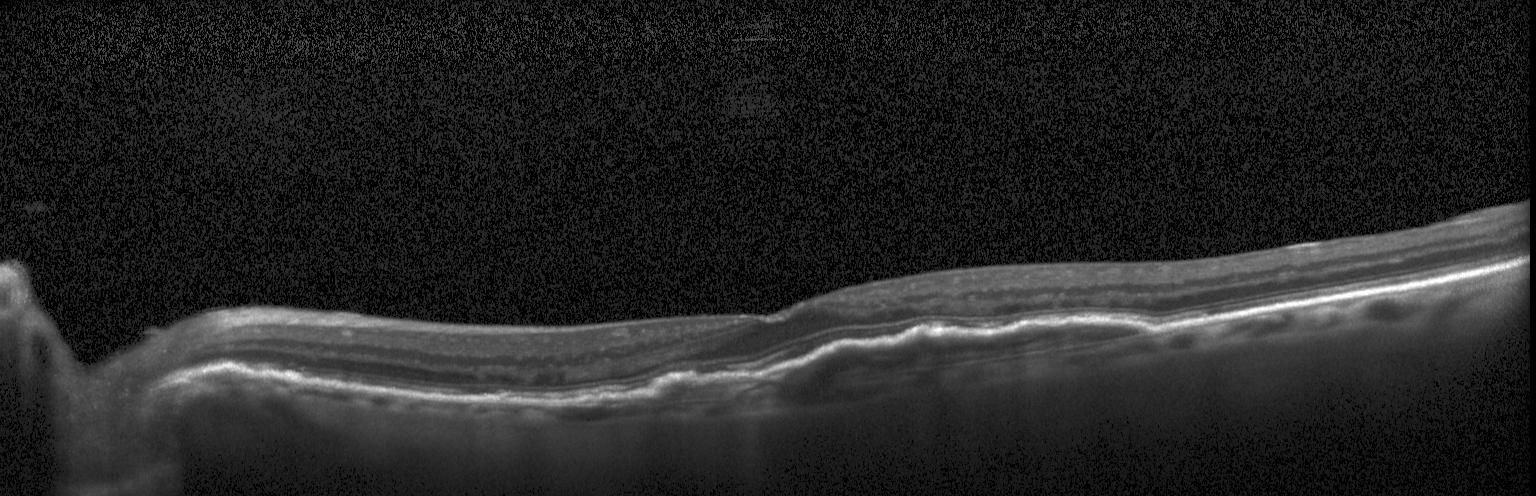 This B-scan demonstrates choroidal neovascularization.